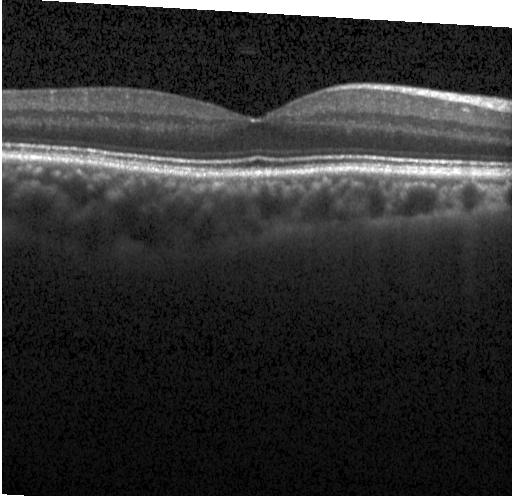
Through the macula, optical coherence tomography scan
Impression: neither choroidal neovascularization, diabetic macular edema, nor drusen.